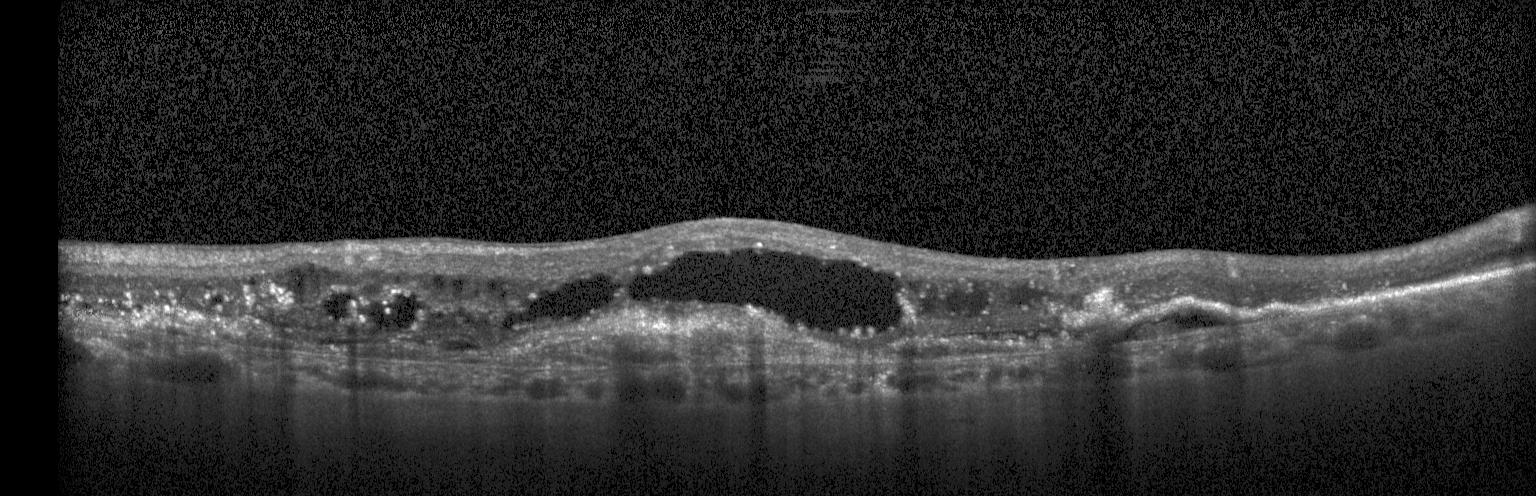 OCT B-scan — Finding: a choroidal neovascular membrane.